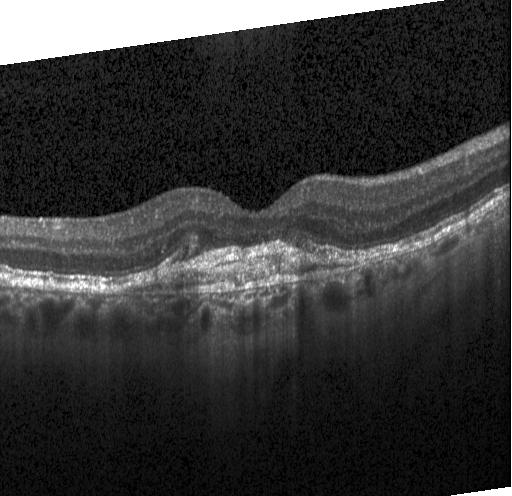
Retinal OCT cross-section · Heidelberg Spectralis OCT system. Finding: CNV.